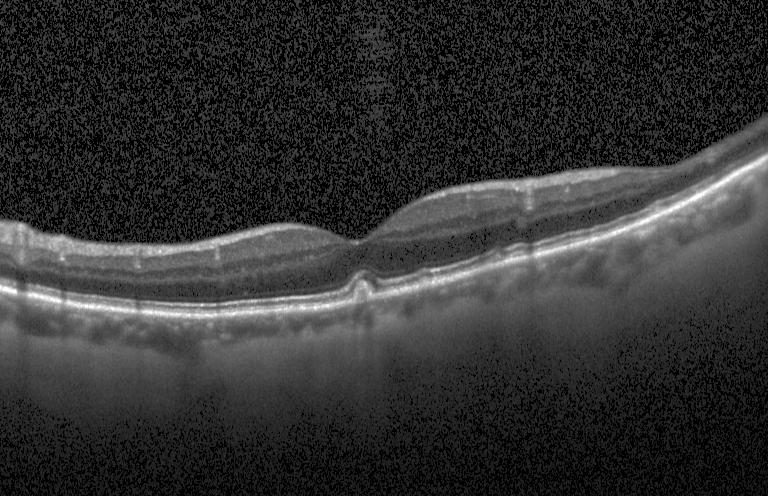 Fovea-centered · retinal OCT B-scan — Diagnosis: sub-RPE drusenoid deposits.